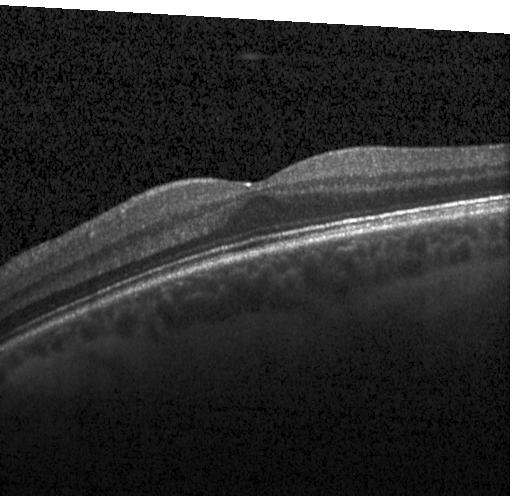
Impression: no choroidal neovascularization, diabetic macular edema, or drusen.